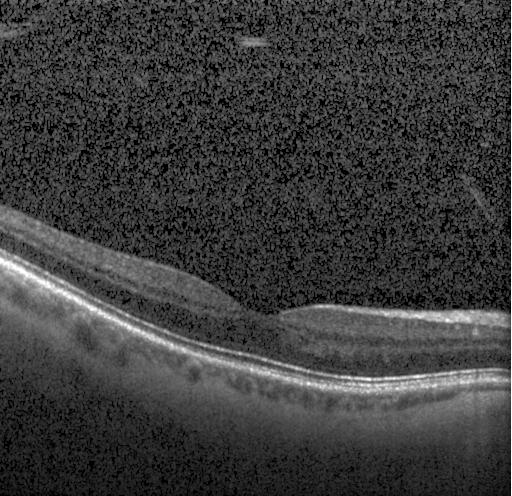

Dx: neither CNV, DME, nor drusen.